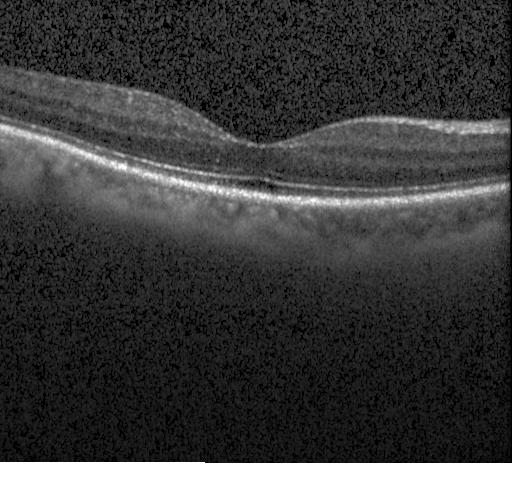 OCT B-scan showing no choroidal neovascularization, diabetic macular edema, or drusen.